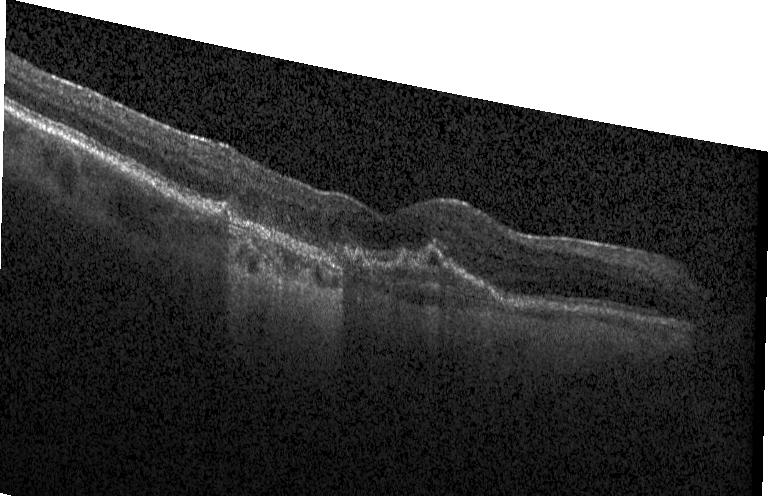
OCT B-scan, SD-OCT, through the macula, instrument: Heidelberg Spectralis. Impression: choroidal neovascularization (CNV).